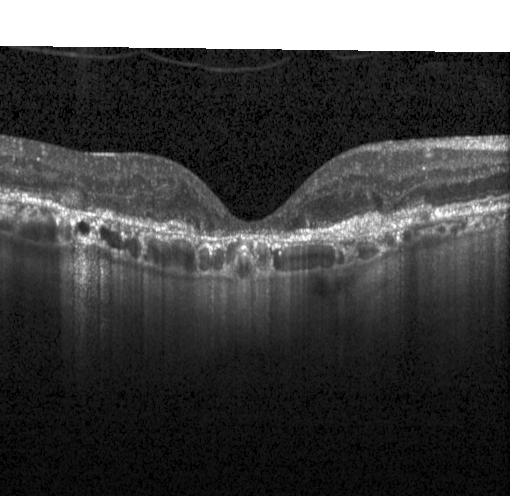 Heidelberg Spectralis; optical coherence tomography B-scan; spectral-domain optical coherence tomography — Impression: CNV.